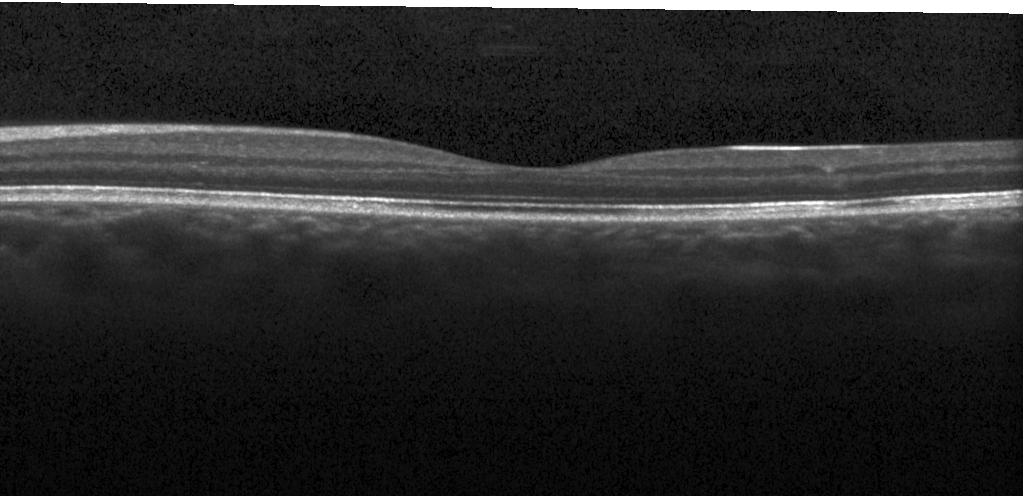
Impression: no CNV, no DME, and no drusen.